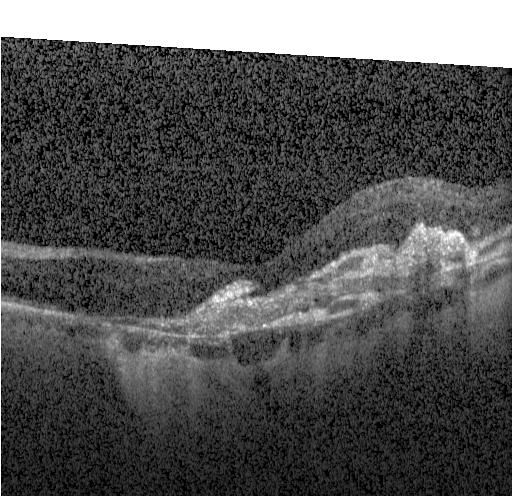
Instrument: Heidelberg Spectralis. Retinal OCT B-scan
Macular OCT: CNV.